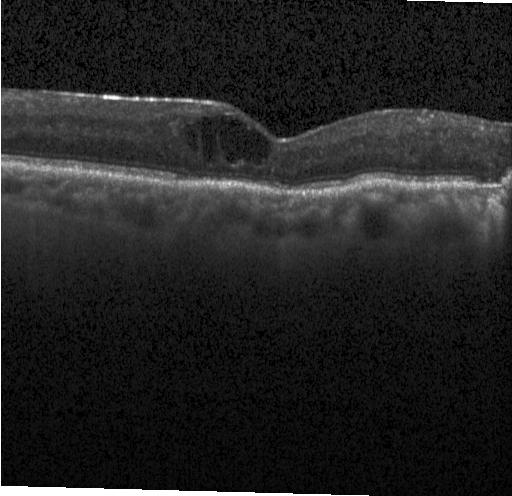 Finding: diabetic macular edema (DME).